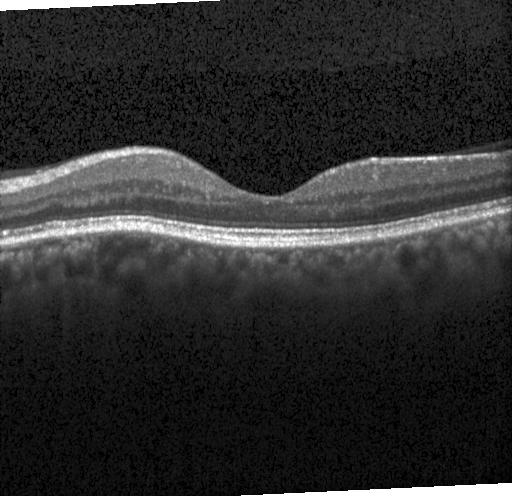

Optical coherence tomography scan. Spectral-domain optical coherence tomography. Acquired on a Heidelberg Spectralis
The scan shows no evidence of choroidal neovascularization, diabetic macular edema, or drusen.